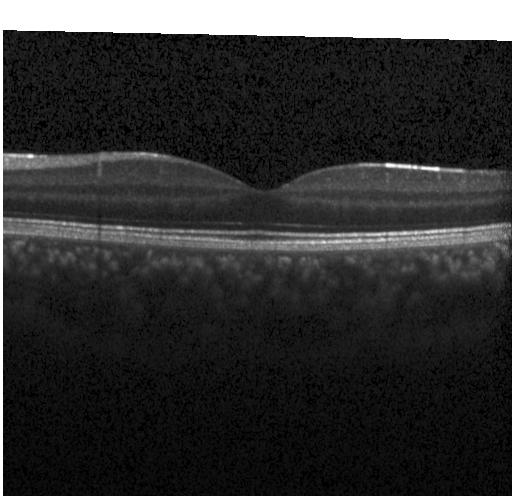

Heidelberg Spectralis OCT system · retinal OCT B-scan · fovea-centered · SD-OCT.
Assessment: neither CNV, DME, nor drusen.